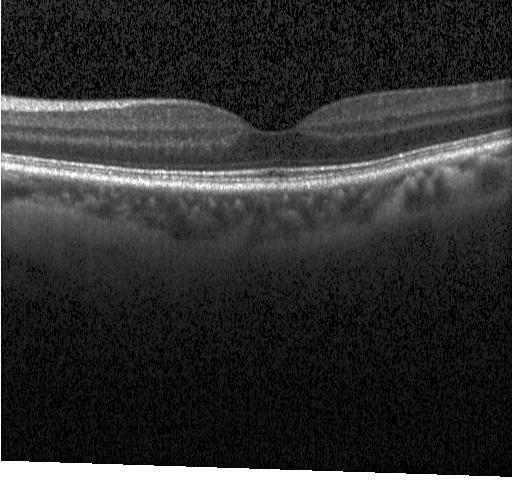

Acquired on a Heidelberg Spectralis. OCT line scan
No choroidal neovascularization, no diabetic macular edema, and no drusen.